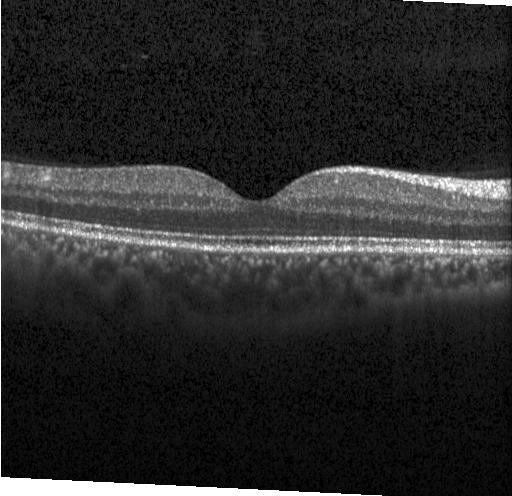

Impression: neither choroidal neovascularization, diabetic macular edema, nor drusen.